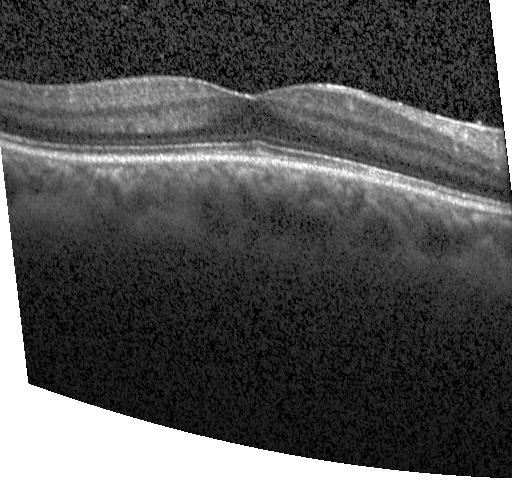

Retinal OCT B-scan. Horizontal scan through the fovea. This B-scan demonstrates no choroidal neovascularization, no diabetic macular edema, and no drusen.